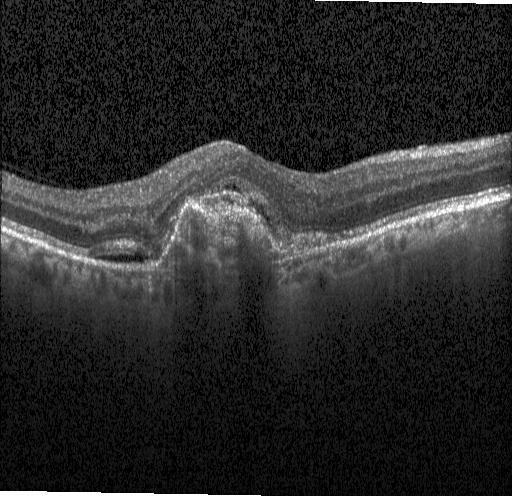

OCT B-scan, Heidelberg Spectralis, SD-OCT — Macular OCT: a choroidal neovascular membrane.